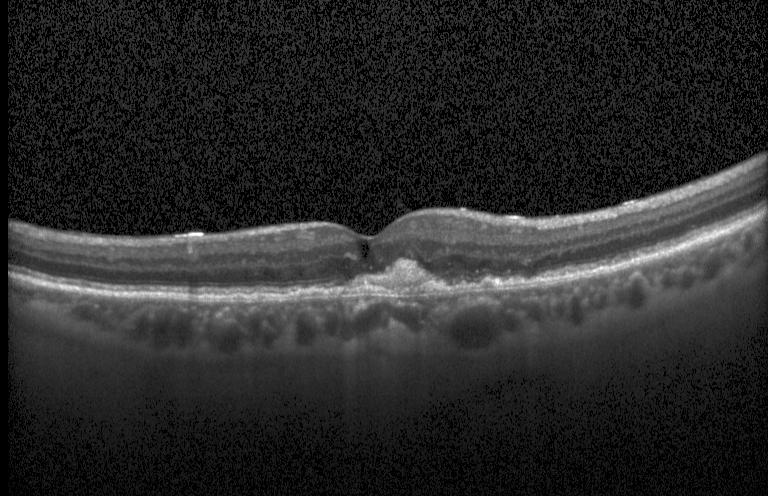 Retinal OCT cross-section
Impression: a choroidal neovascular membrane.